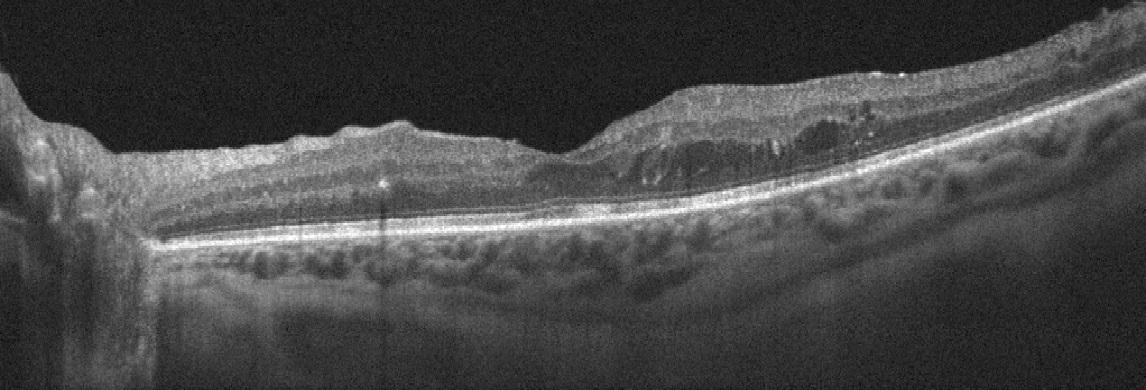
Fovea-centered. OCT line scan. Acquired on an Optovue Avanti RTVue XR.
Diagnosis: DME.